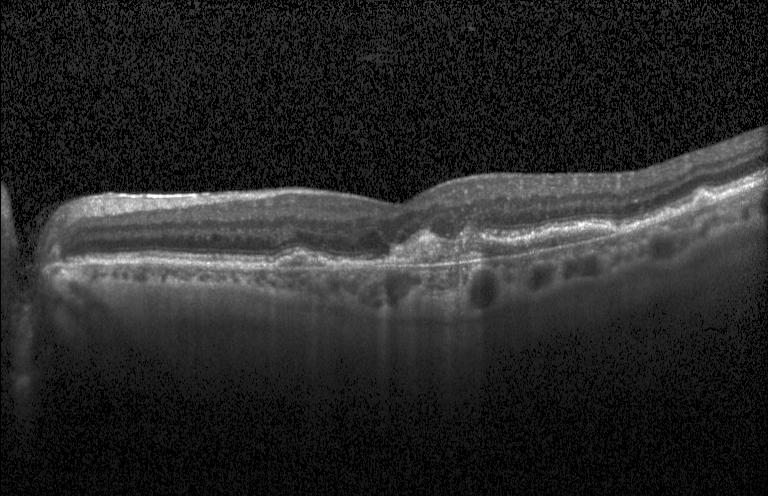

Retinal OCT B-scan; horizontal scan through the fovea; instrument: Heidelberg Spectralis; spectral-domain optical coherence tomography.
Dx: a choroidal neovascular membrane.